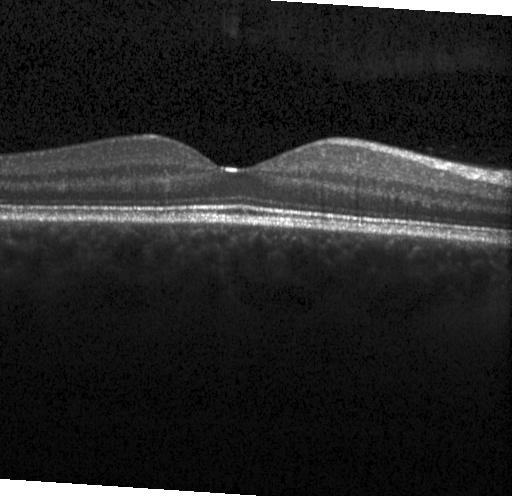
Spectral-domain OCT, optical coherence tomography B-scan, instrument: Heidelberg Spectralis, horizontal scan through the fovea. Impression: no choroidal neovascularization, diabetic macular edema, or drusen.